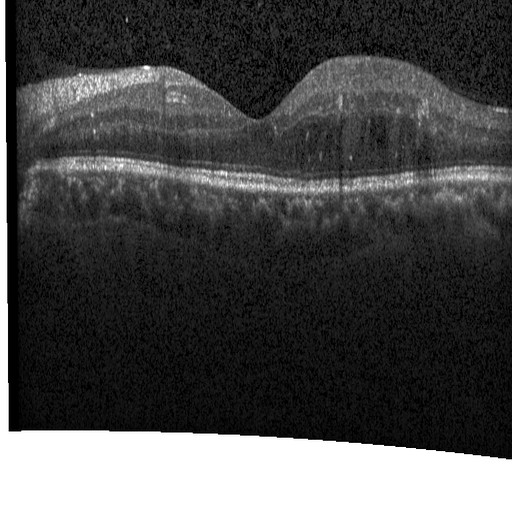 Impression: DME.